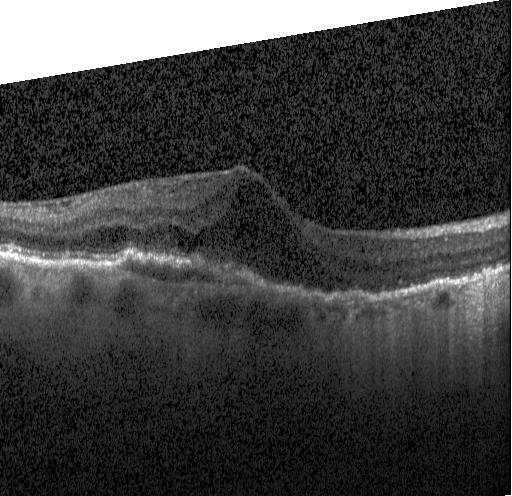 Heidelberg Spectralis · macular scan · OCT line scan. Finding: choroidal neovascularization.